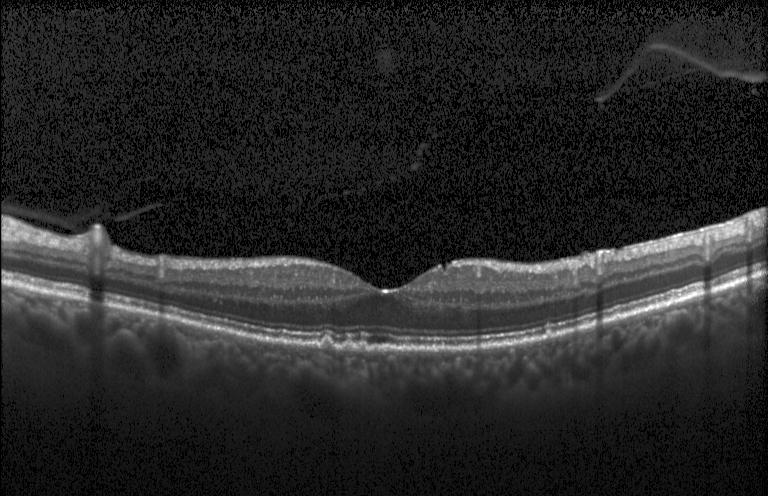
OCT line scan · Heidelberg Spectralis OCT system · horizontal scan through the fovea · SD-OCT. Drusen.